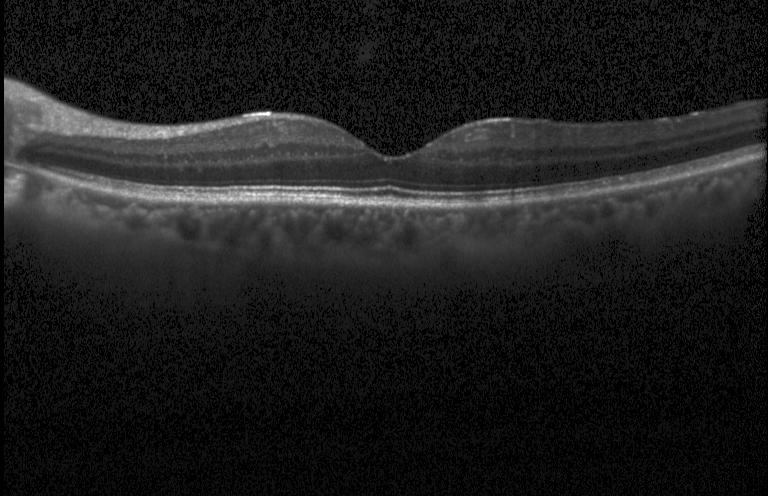
Retinal OCT B-scan
Diagnosis: no choroidal neovascularization, diabetic macular edema, or drusen.